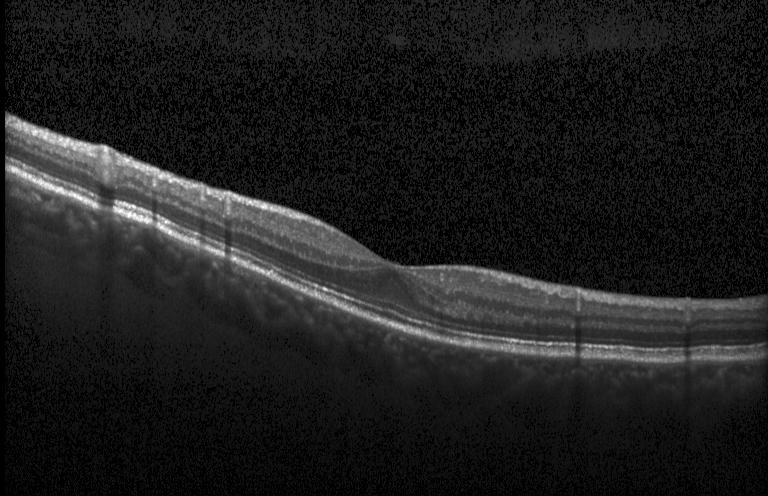
Optical coherence tomography scan — Dx: no choroidal neovascularization, diabetic macular edema, or drusen.